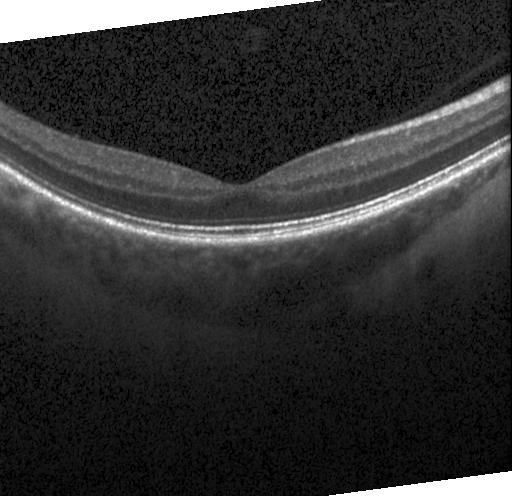

Dx: no choroidal neovascularization, no diabetic macular edema, and no drusen.